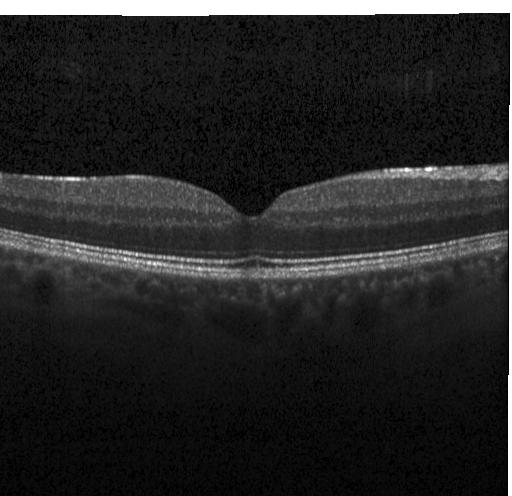 Optical coherence tomography B-scan, centered on the fovea — OCT finding: neither choroidal neovascularization, diabetic macular edema, nor drusen.